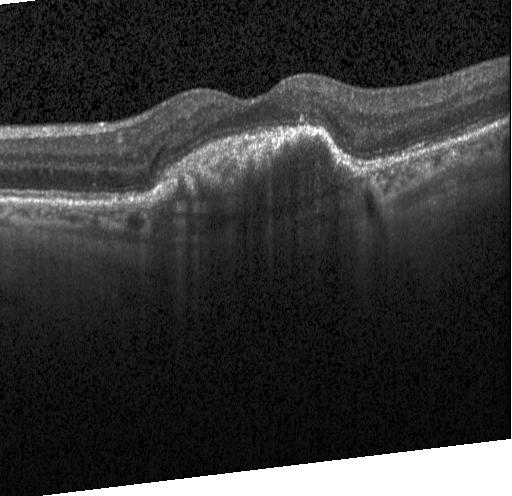 Optical coherence tomography B-scan — Diagnosis: a choroidal neovascular membrane.